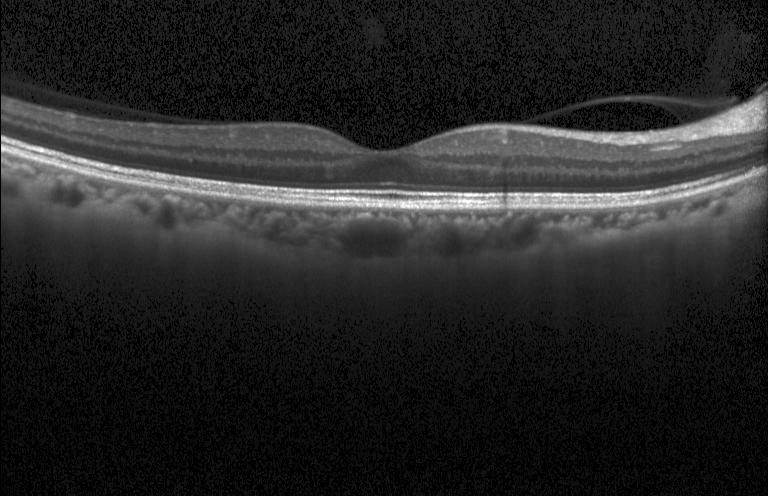
OCT B-scan showing neither CNV, DME, nor drusen.